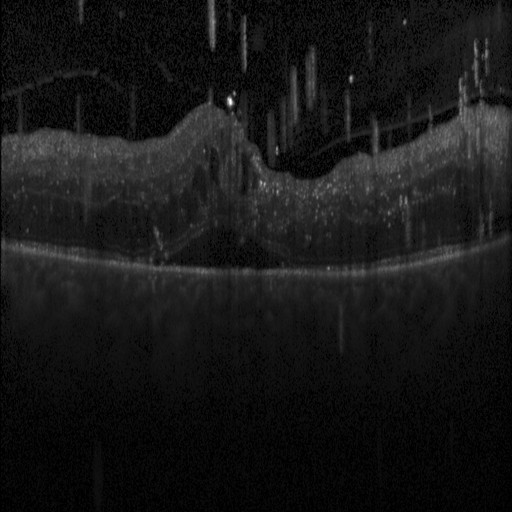

The scan shows diabetic macular edema (DME).